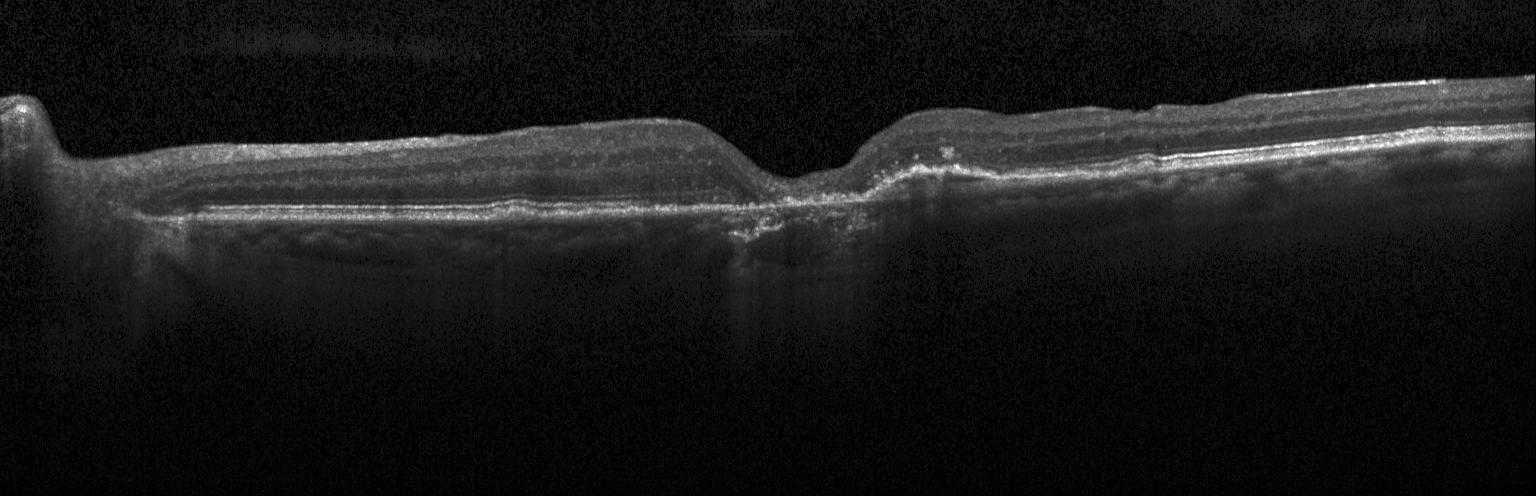
A choroidal neovascular membrane.